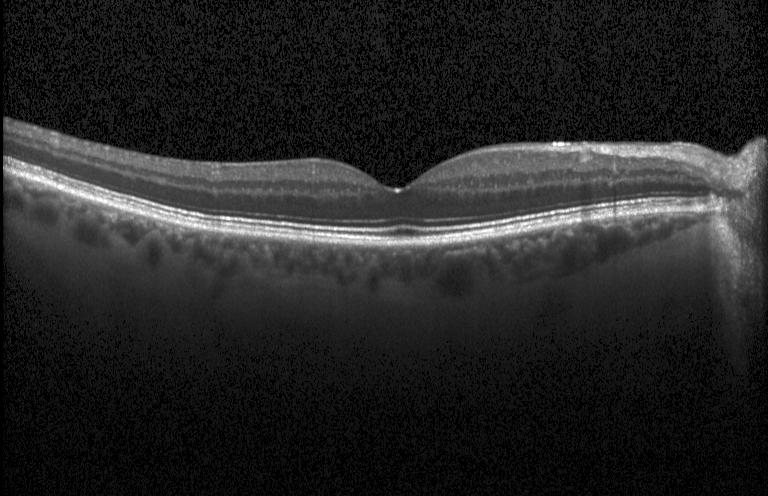 Impression: no evidence of CNV, DME, or drusen.